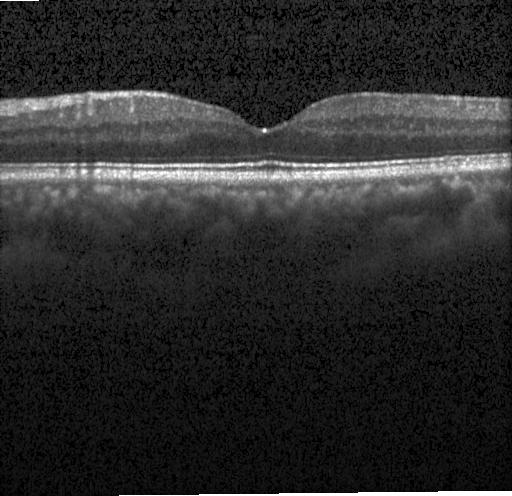

OCT scan showing no choroidal neovascularization, diabetic macular edema, or drusen.